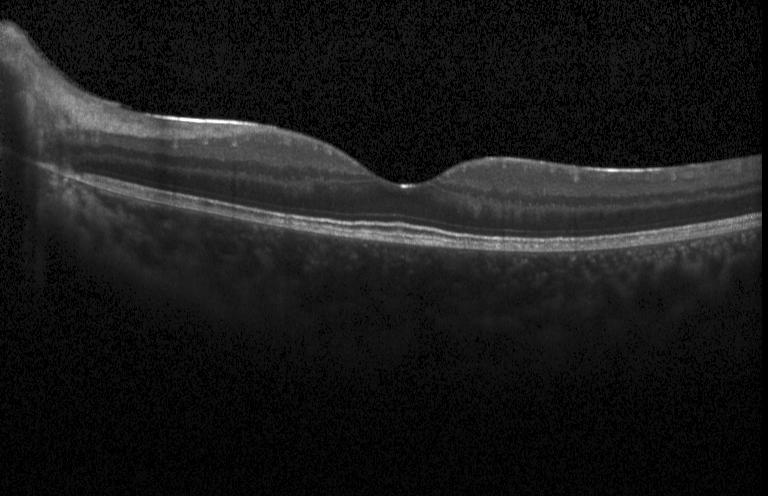

Spectral-domain OCT B-scan: neither choroidal neovascularization, diabetic macular edema, nor drusen.